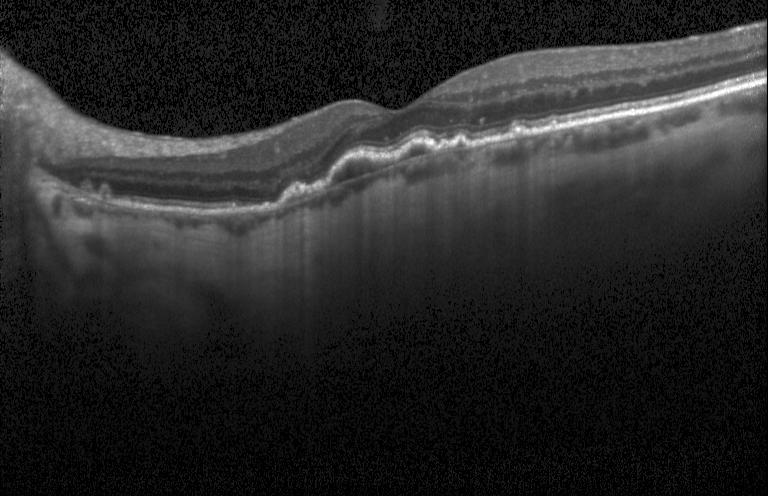
Fovea-centered · SD-OCT · Heidelberg Spectralis OCT system · retinal OCT B-scan.
Assessment: CNV.